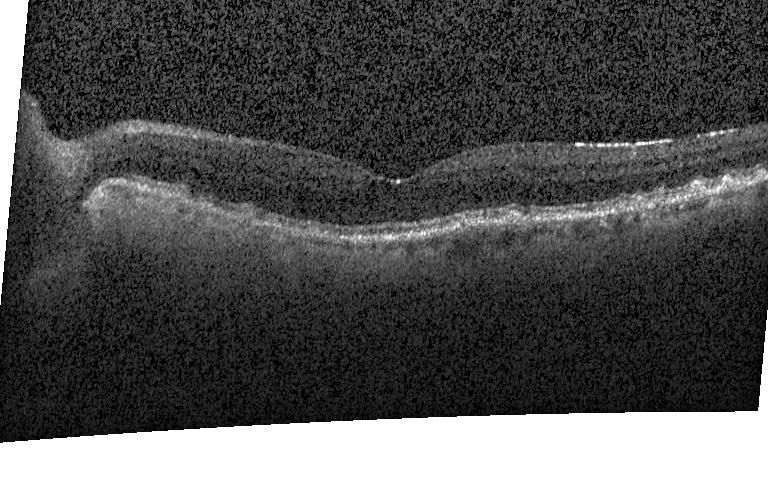
Spectral-domain optical coherence tomography, horizontal scan through the fovea, OCT B-scan — Assessment: sub-RPE drusenoid deposits.